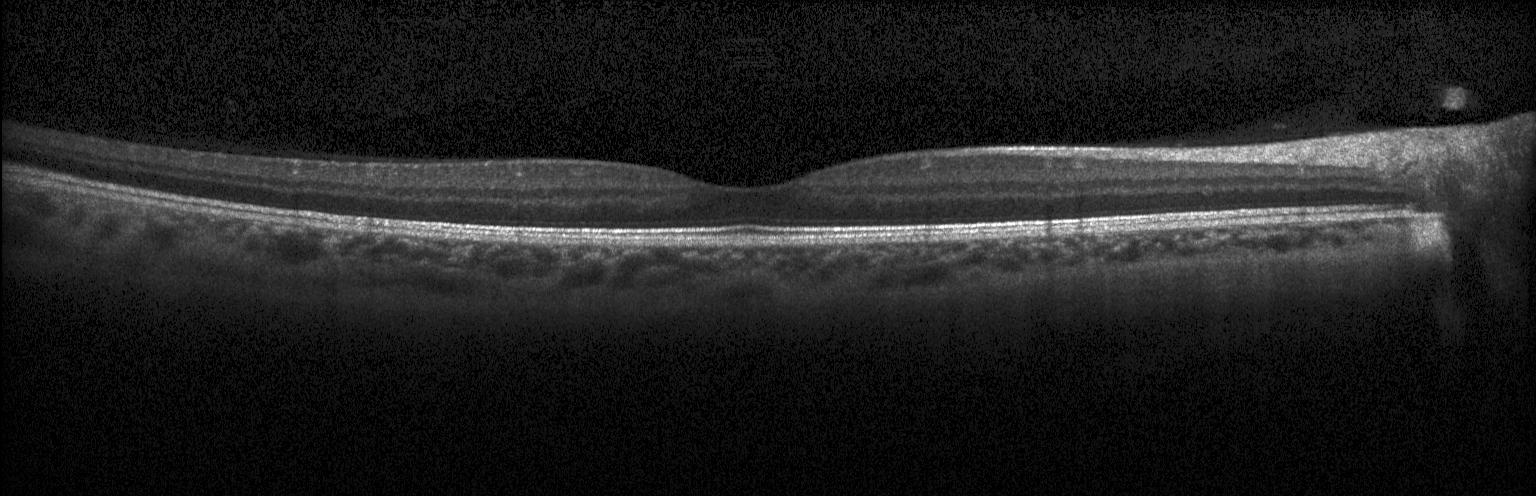 Optical coherence tomography scan · SD-OCT · through the macula. Finding: no choroidal neovascularization, no diabetic macular edema, and no drusen.